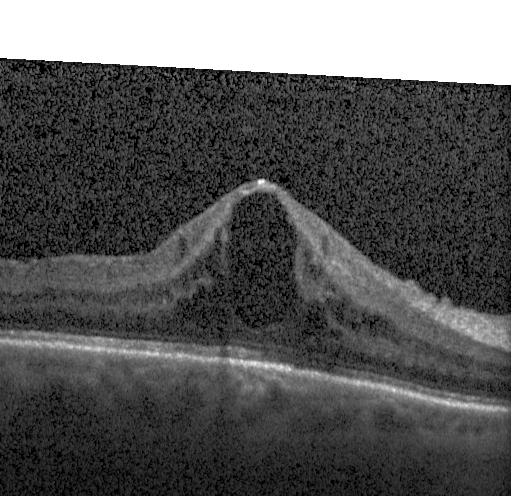

Optical coherence tomography scan.
Finding: DME.